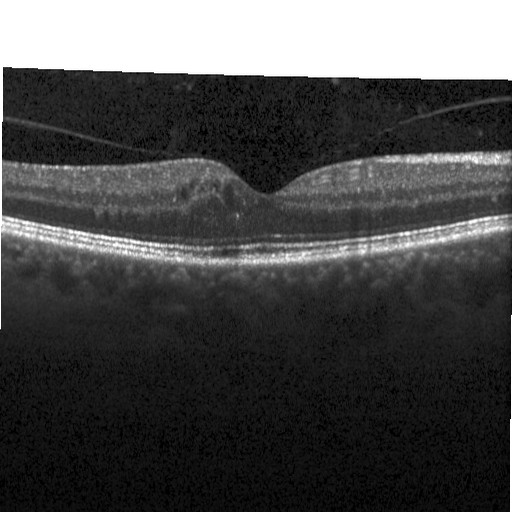 Optical coherence tomography scan, spectral-domain OCT, acquired on a Heidelberg Spectralis
Diagnosis: diabetic macular edema (DME).